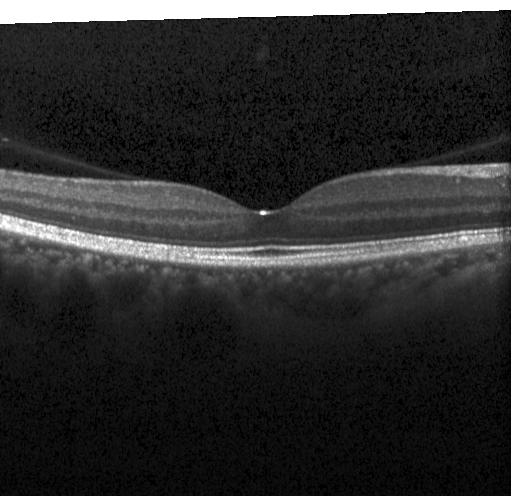

Optical coherence tomography scan. OCT finding: no CNV, no DME, and no drusen.